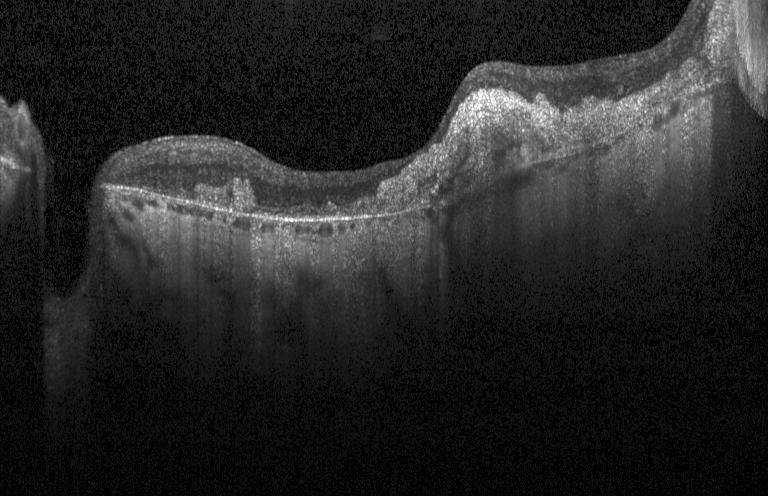

Optical coherence tomography B-scan.
Diagnosis: choroidal neovascularization (CNV).